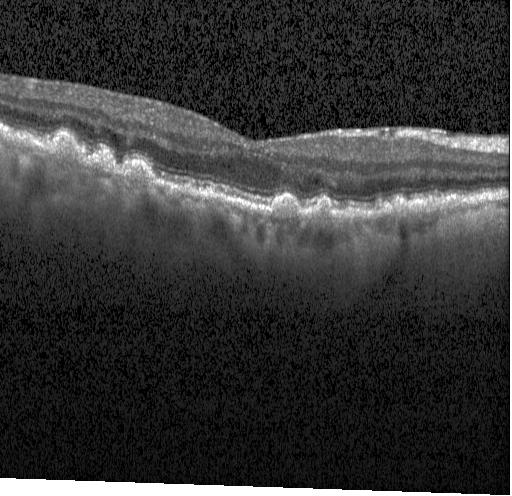

Finding: sub-RPE drusenoid deposits.